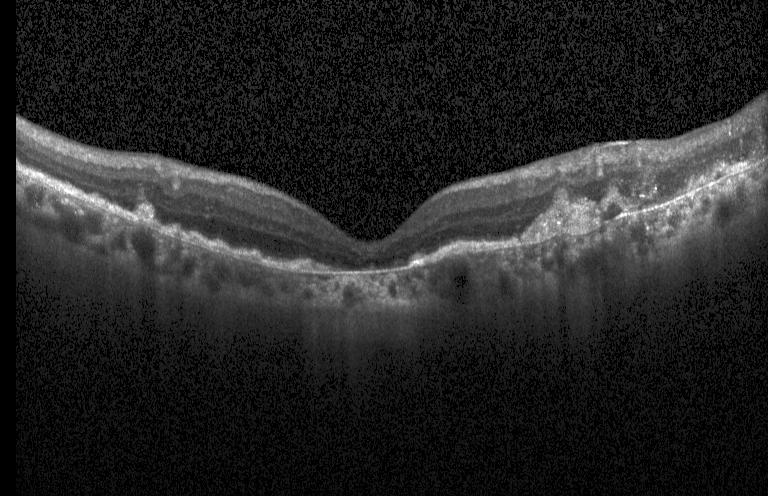

Fovea-centered. Retinal OCT B-scan.
Macular OCT: a choroidal neovascular membrane.